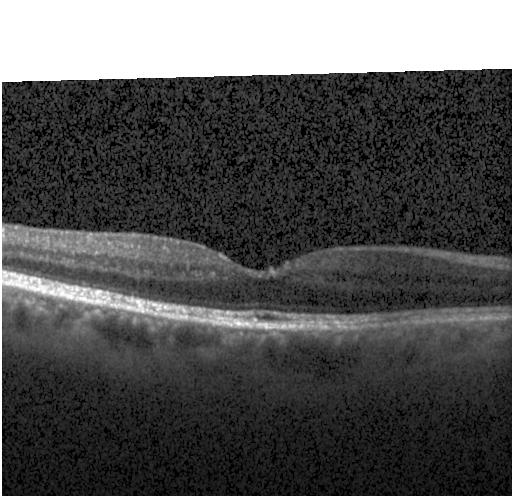
Centered on the fovea. OCT line scan.
Macular OCT: no CNV, DME, or drusen.